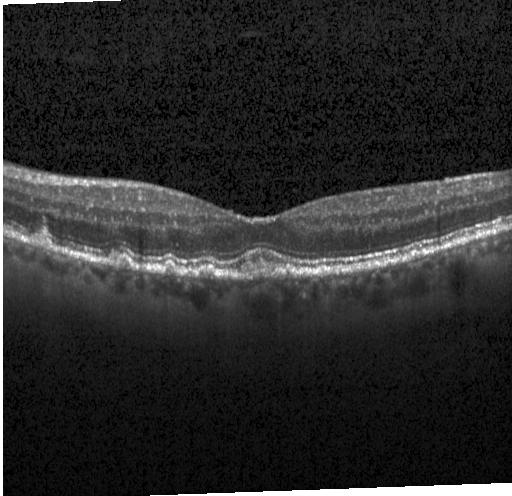

Optical coherence tomography B-scan · instrument: Heidelberg Spectralis · through the macula.
OCT finding: multiple drusen.